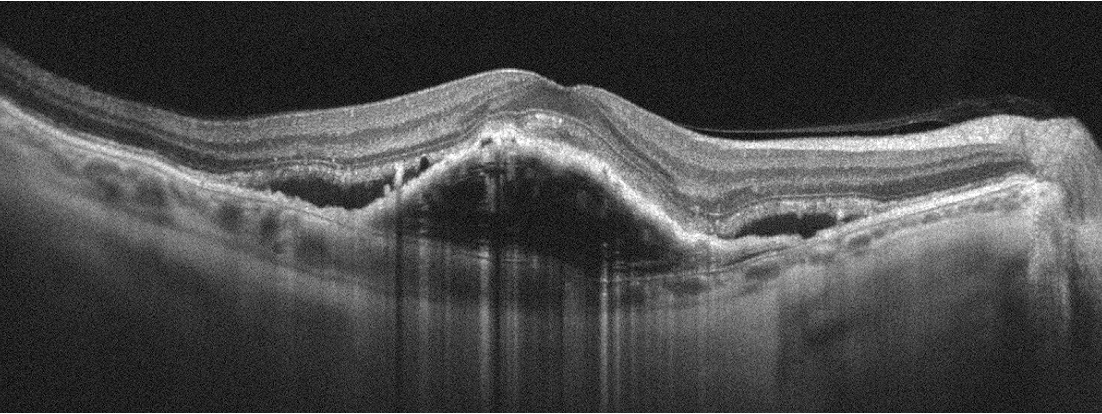

Optical coherence tomography B-scan · Optovue Avanti RTVue XR · fovea-centered — The scan shows age-related macular degeneration.